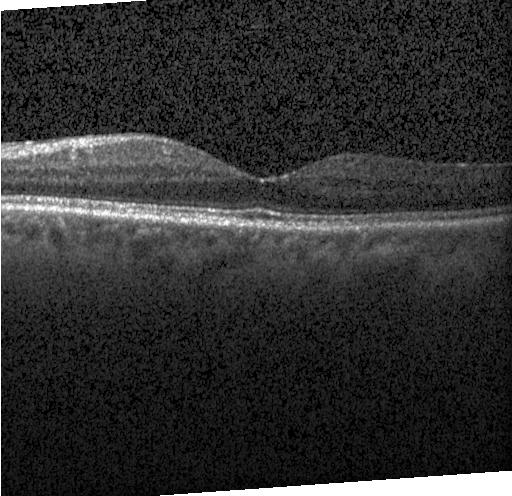
Retinal OCT cross-section showing no CNV, no DME, and no drusen.